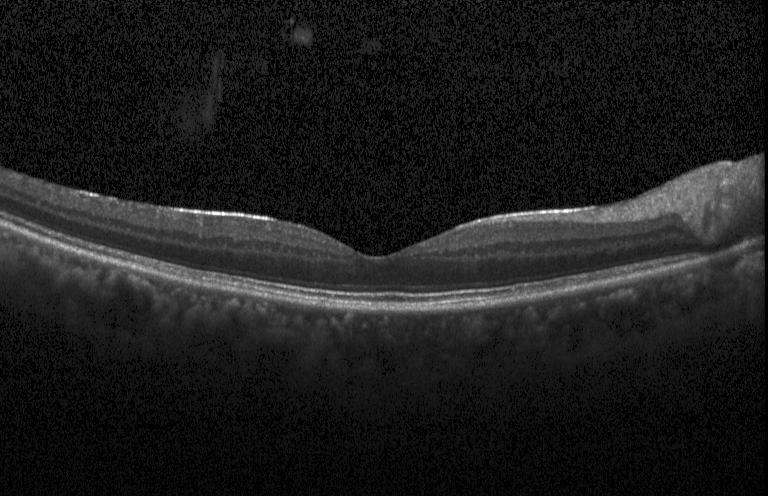

Spectral-domain OCT, horizontal scan through the fovea, Heidelberg Spectralis OCT system, optical coherence tomography B-scan
Diagnosis: no choroidal neovascularization, diabetic macular edema, or drusen.